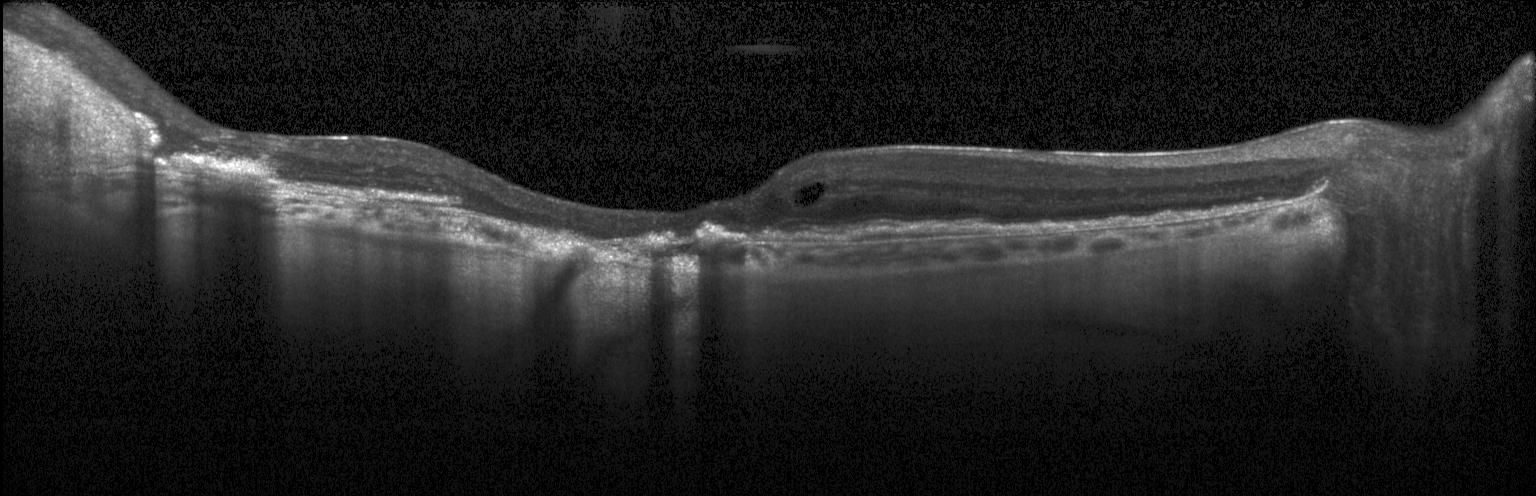 Optical coherence tomography scan. Through the macula
This B-scan demonstrates CNV.